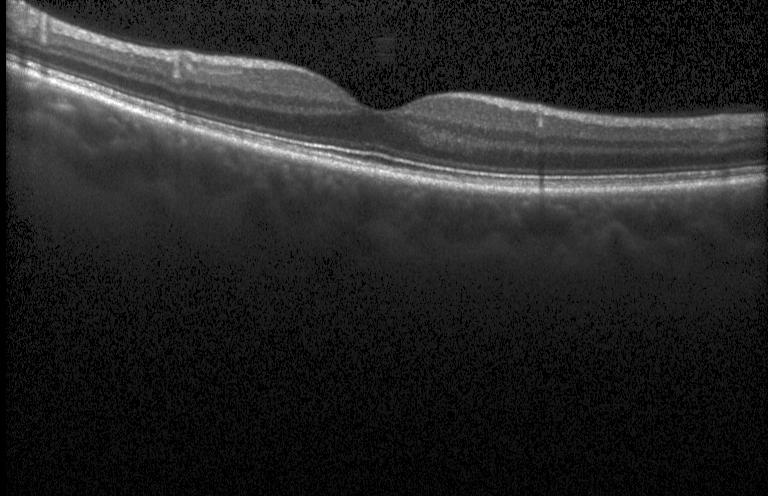

Retinal OCT B-scan; horizontal scan through the fovea — Macular OCT: no CNV, DME, or drusen.